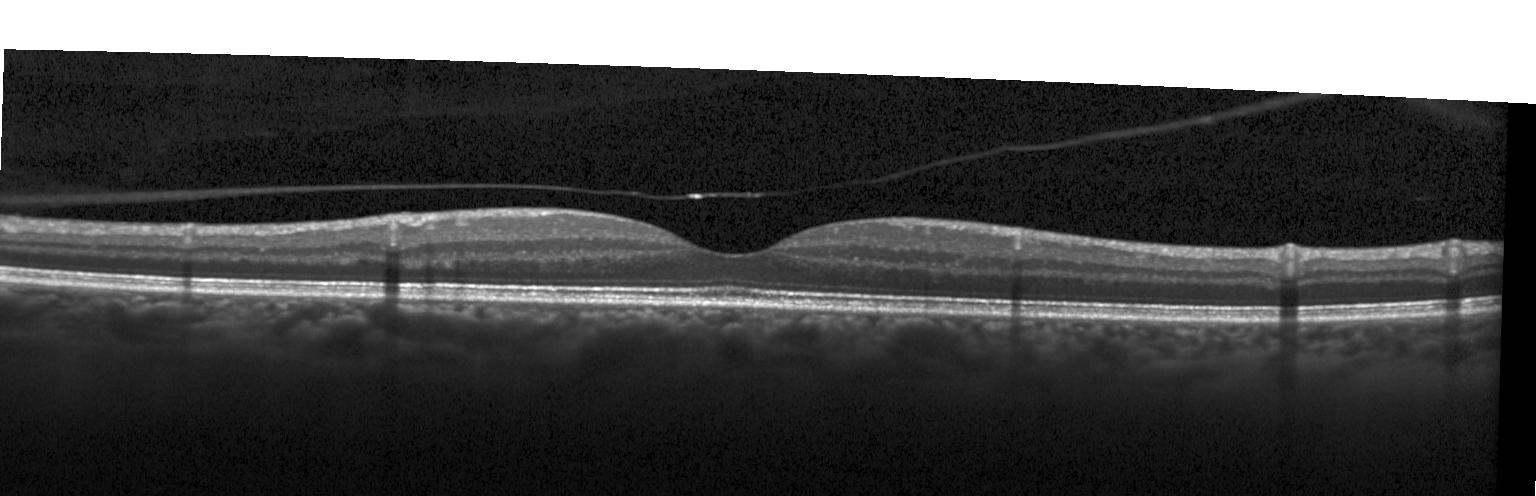

Impression: no choroidal neovascularization, diabetic macular edema, or drusen.